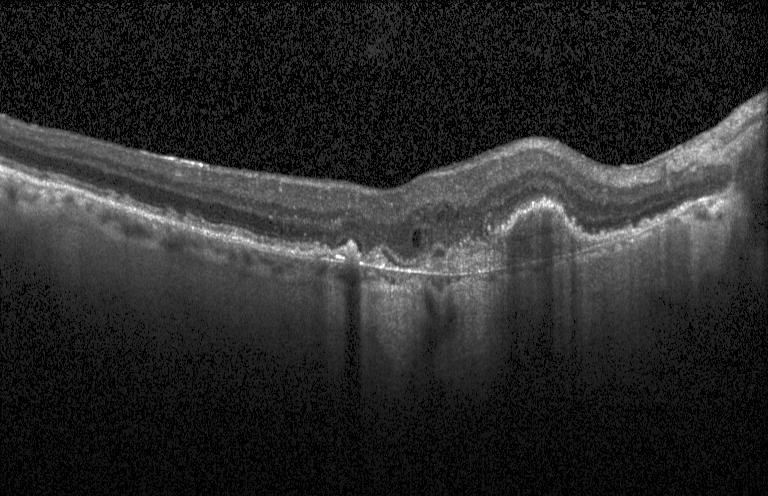

Instrument: Heidelberg Spectralis. SD-OCT. Retinal OCT B-scan. Centered on the fovea
Diagnosis: choroidal neovascularization.